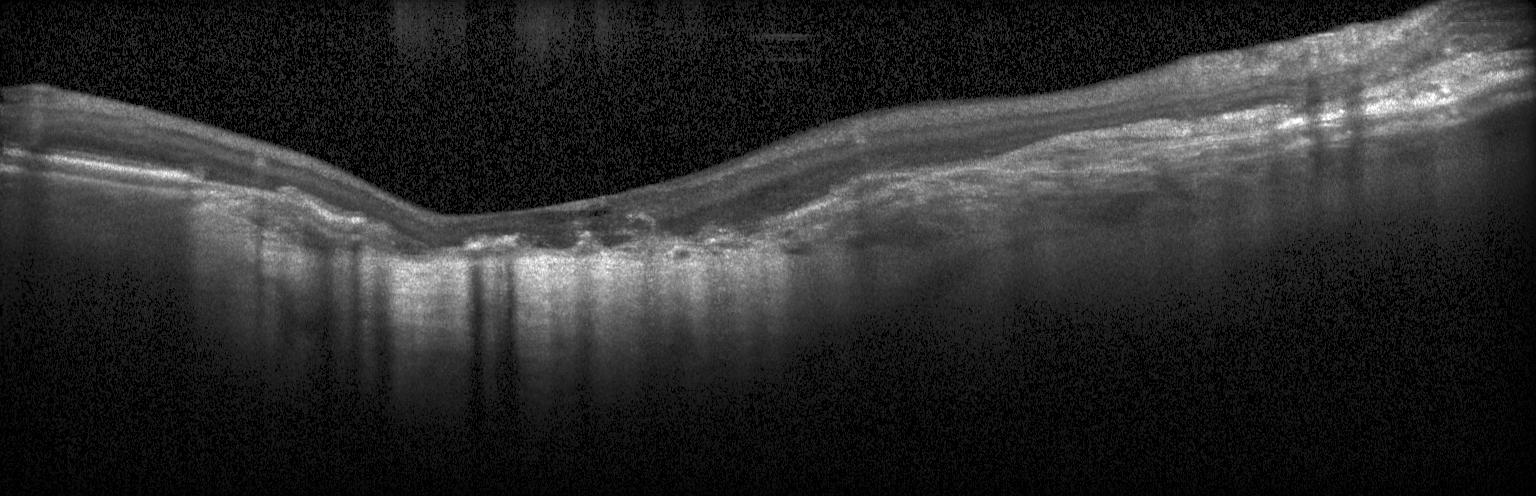 Heidelberg Spectralis. Optical coherence tomography B-scan.
Dx: choroidal neovascularization (CNV).